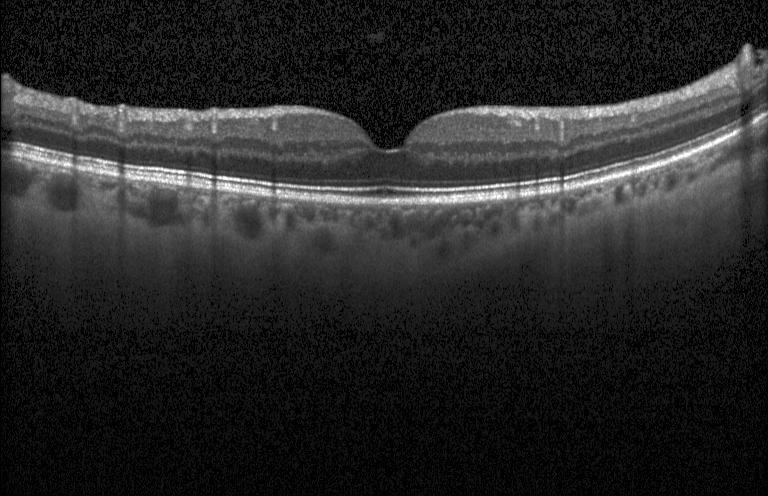 Neither choroidal neovascularization, diabetic macular edema, nor drusen.